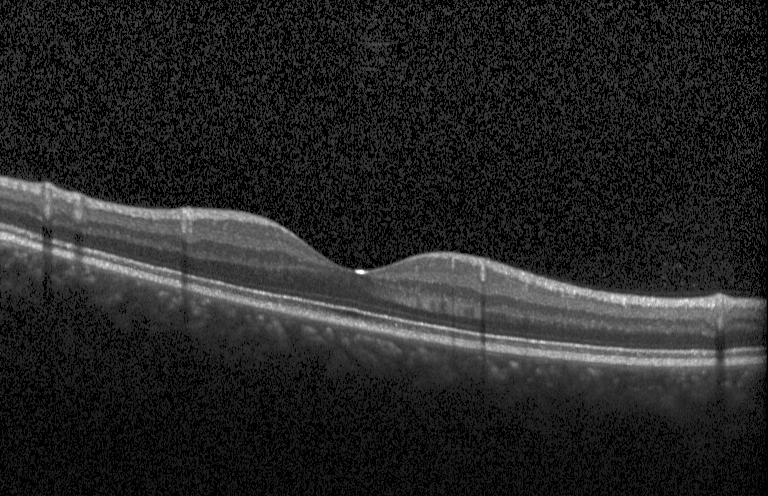 OCT finding: neither choroidal neovascularization, diabetic macular edema, nor drusen.